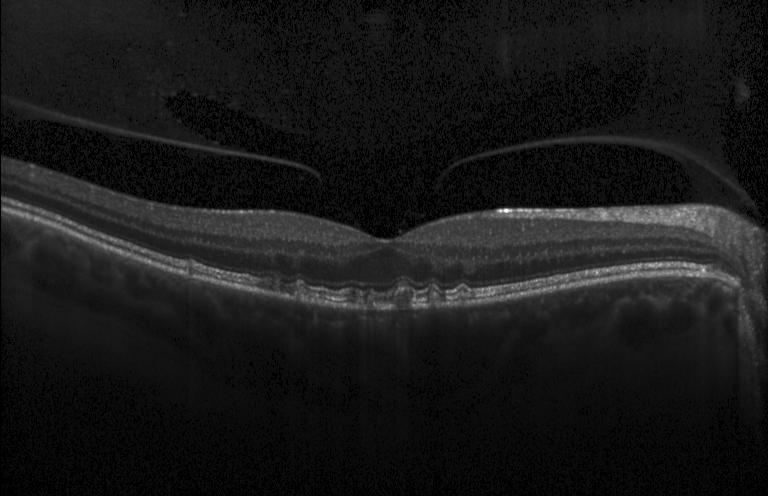
This B-scan demonstrates multiple drusen.